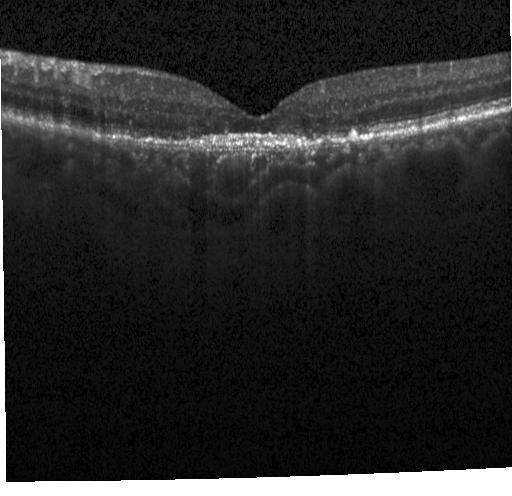 Dx: a choroidal neovascular membrane.